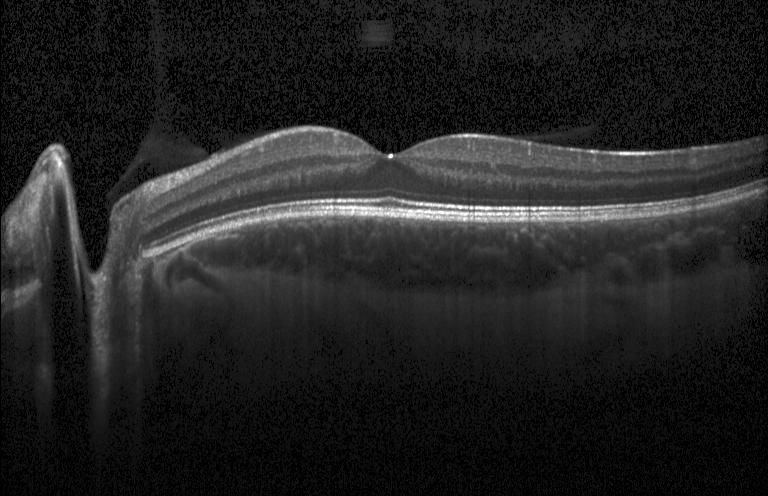 The scan shows no choroidal neovascularization, diabetic macular edema, or drusen.